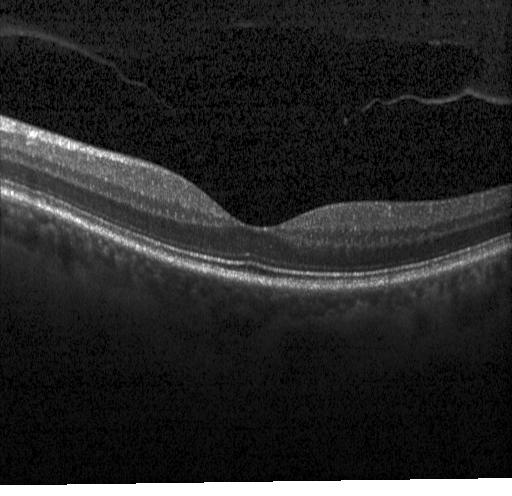

Macular OCT demonstrating no choroidal neovascularization, diabetic macular edema, or drusen.